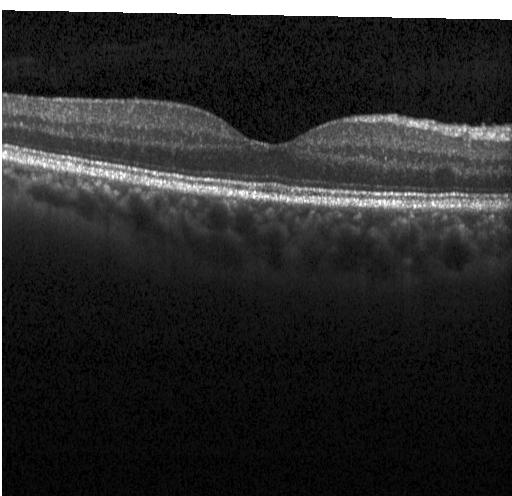 No evidence of choroidal neovascularization, diabetic macular edema, or drusen.